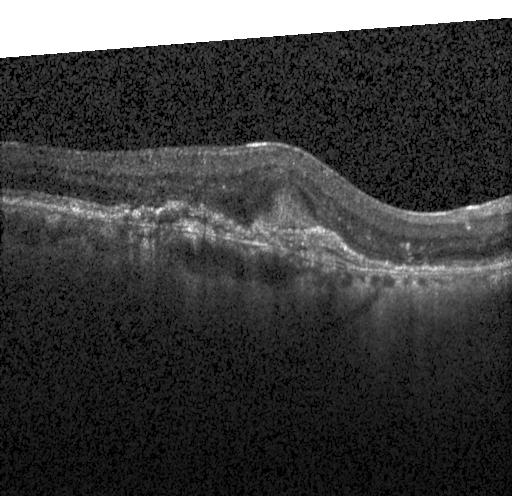 OCT B-scan, spectral-domain optical coherence tomography, acquired on a Heidelberg Spectralis, centered on the fovea.
The scan shows choroidal neovascularization.